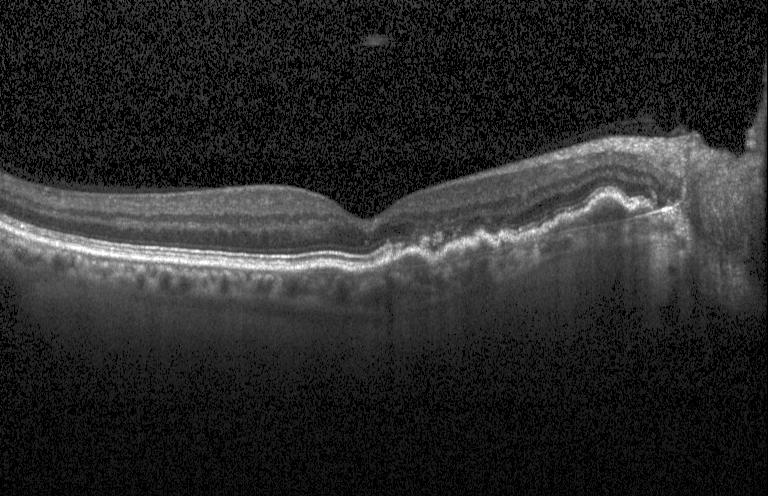
Spectral-domain OCT, optical coherence tomography B-scan — A choroidal neovascular membrane.